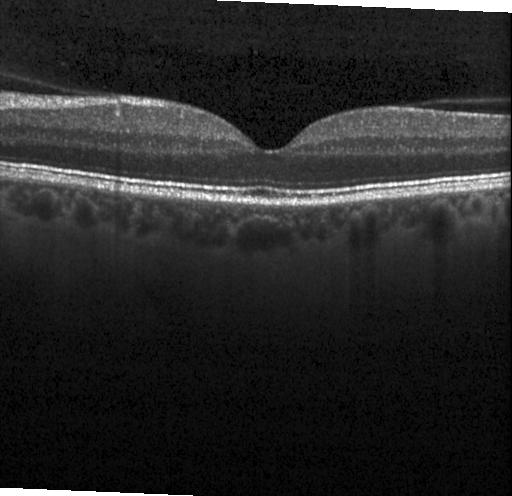 Spectral-domain OCT B-scan: no choroidal neovascularization, no diabetic macular edema, and no drusen.